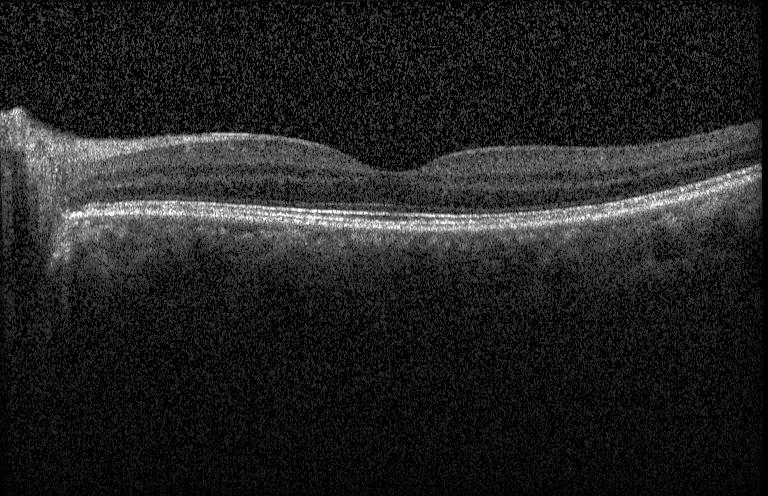 Retinal OCT cross-section · instrument: Heidelberg Spectralis · spectral-domain OCT.
No evidence of choroidal neovascularization, diabetic macular edema, or drusen.